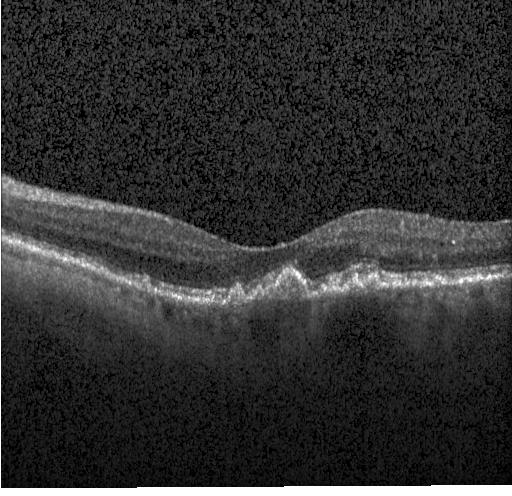 Finding: multiple drusen.